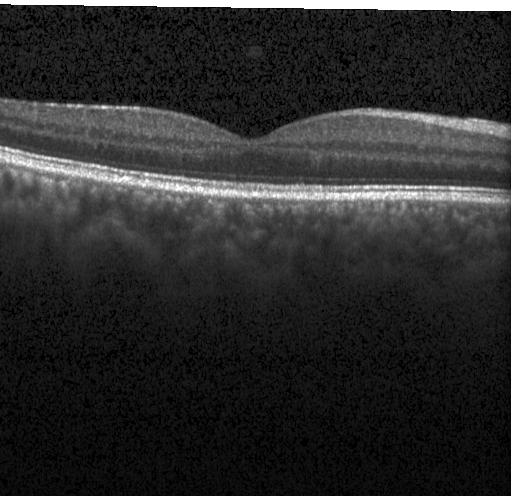
Optical coherence tomography B-scan. SD-OCT.
Impression: no choroidal neovascularization, no diabetic macular edema, and no drusen.